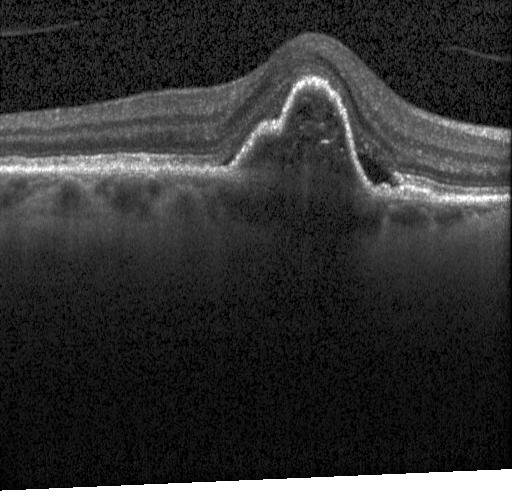 Spectral-domain optical coherence tomography, acquired on a Heidelberg Spectralis, optical coherence tomography B-scan.
Finding: choroidal neovascularization (CNV).